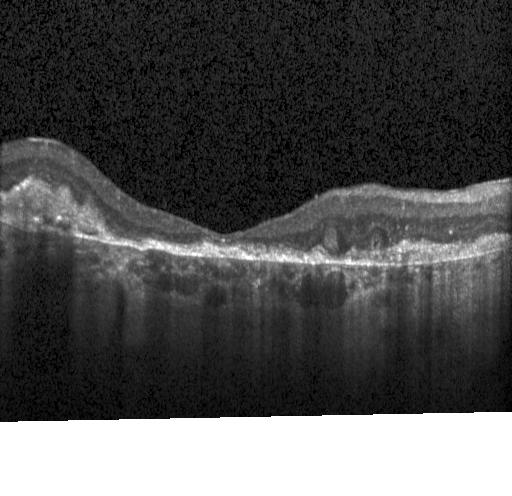

Macular OCT: a choroidal neovascular membrane.